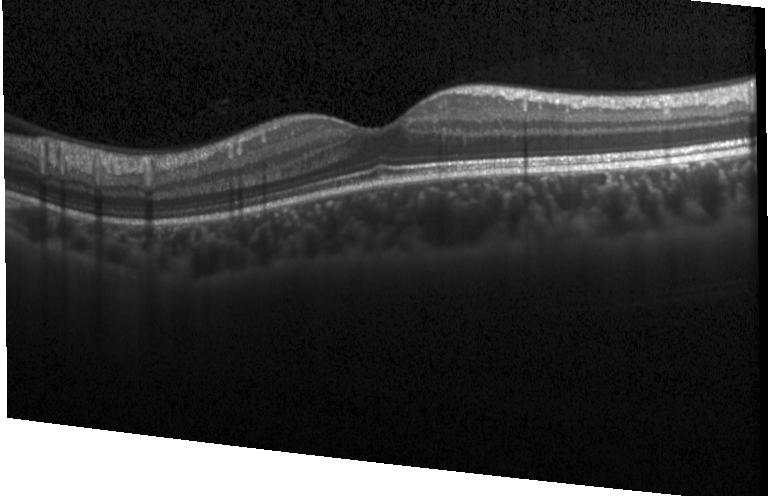
Optical coherence tomography scan, horizontal scan through the fovea.
Finding: no choroidal neovascularization, diabetic macular edema, or drusen.